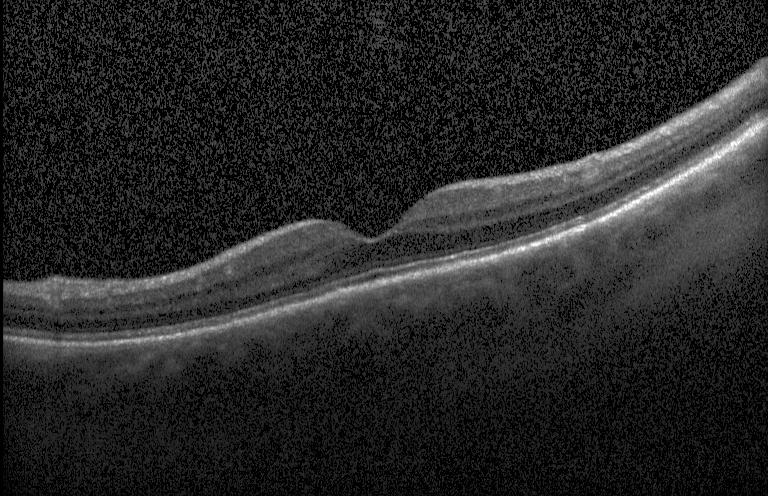 Optical coherence tomography B-scan · fovea-centered · spectral-domain OCT. Impression: no evidence of choroidal neovascularization, diabetic macular edema, or drusen.